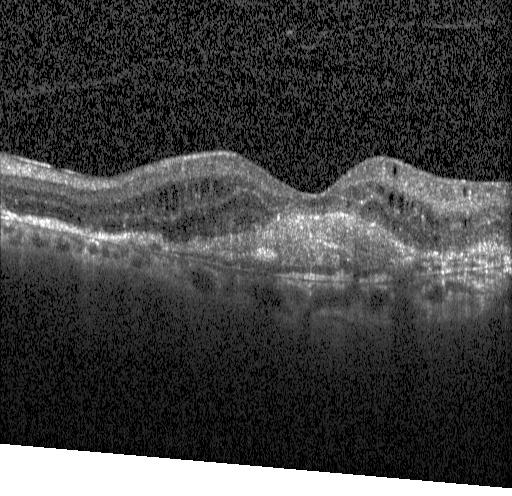 Fovea-centered · optical coherence tomography B-scan — Finding: choroidal neovascularization (CNV).